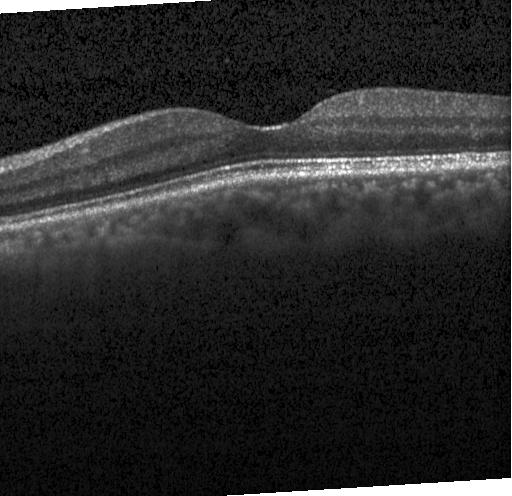 Instrument: Heidelberg Spectralis. Spectral-domain OCT. OCT line scan. Through the macula. This B-scan demonstrates no CNV, DME, or drusen.